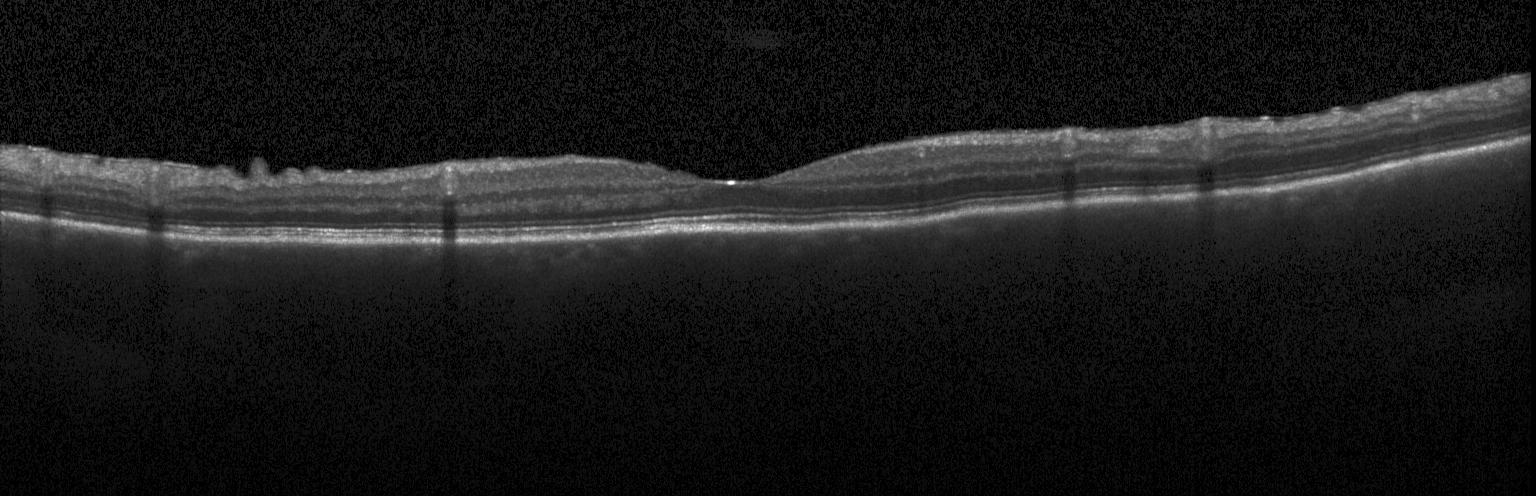
Diagnosis: no choroidal neovascularization, diabetic macular edema, or drusen.